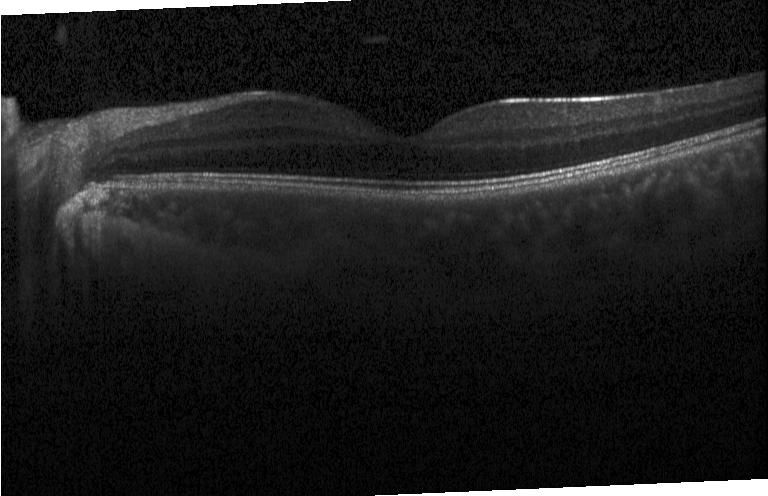
Spectral-domain optical coherence tomography. Optical coherence tomography B-scan. Through the macula. Impression: neither choroidal neovascularization, diabetic macular edema, nor drusen.